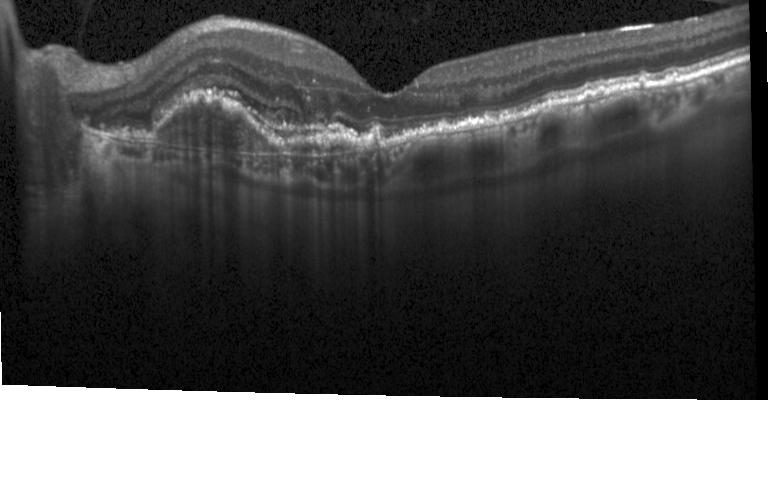 Diagnosis: a choroidal neovascular membrane.